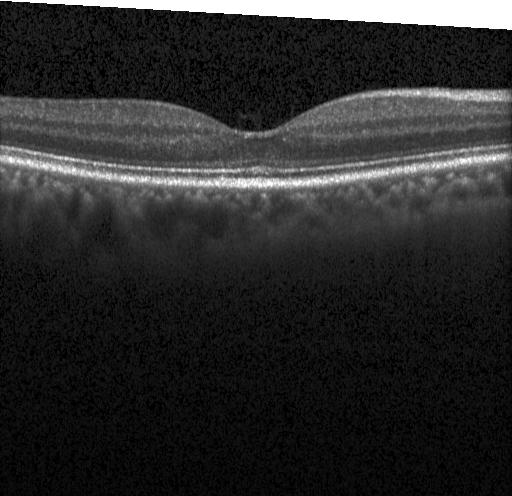
OCT line scan. Spectral-domain OCT. Finding: neither choroidal neovascularization, diabetic macular edema, nor drusen.